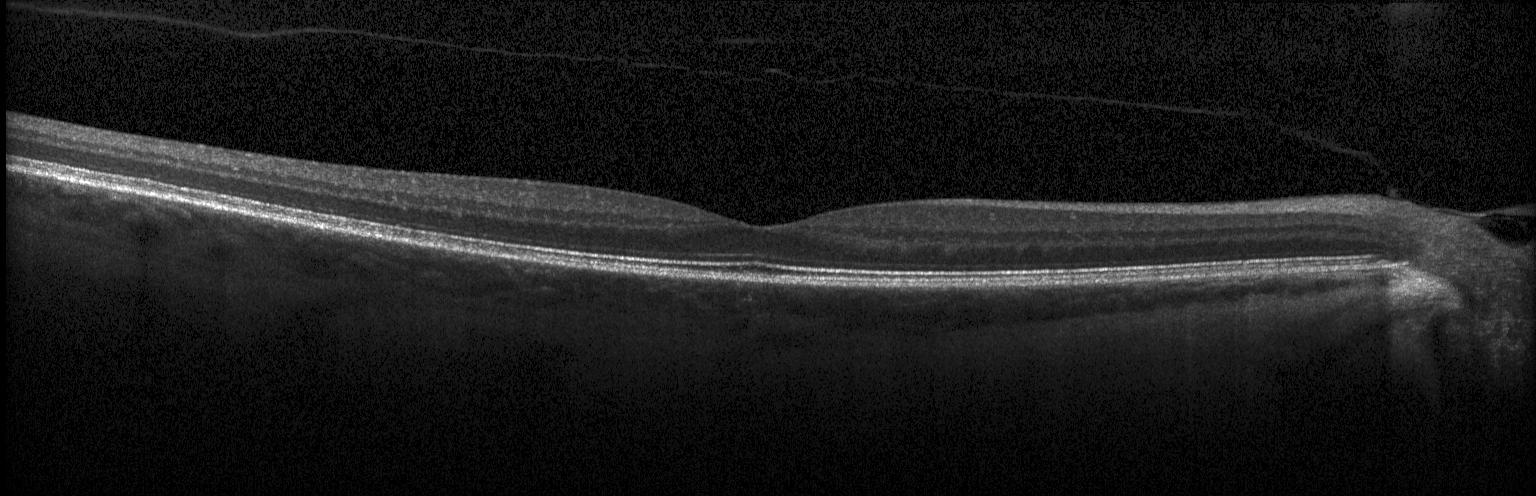
Assessment: no evidence of CNV, DME, or drusen.